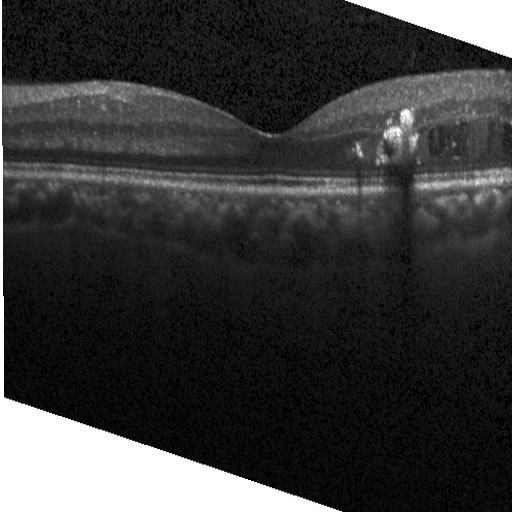
Acquired on a Heidelberg Spectralis, macular scan, OCT line scan, spectral-domain OCT.
The scan shows DME.